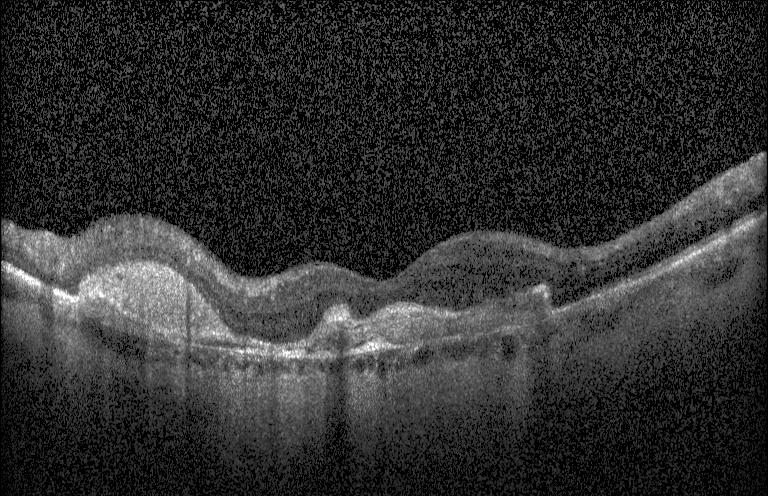
Impression: a choroidal neovascular membrane.